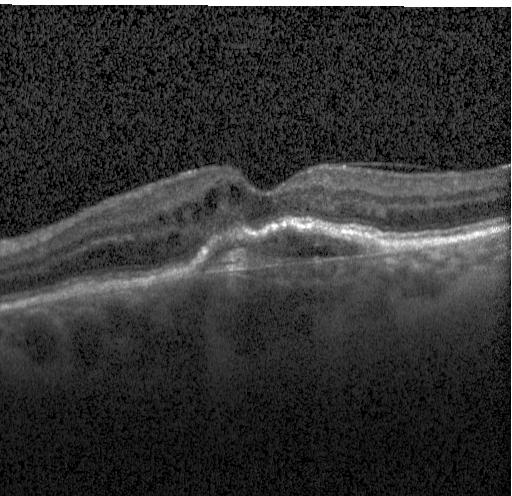 OCT finding: a choroidal neovascular membrane.